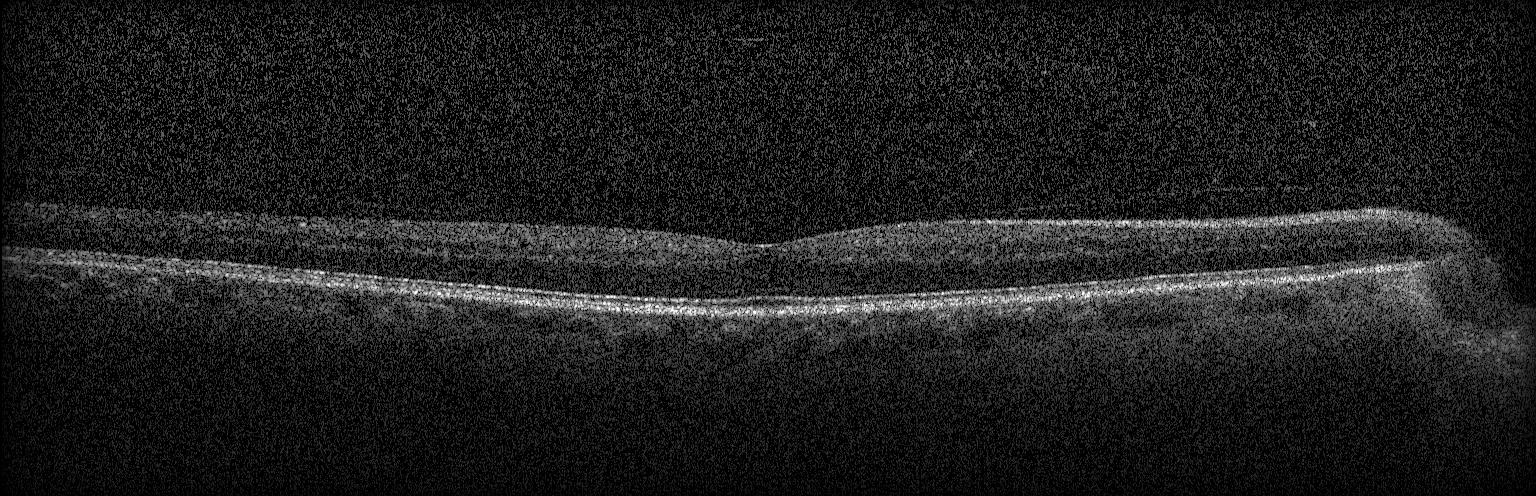
OCT B-scan · through the macula · Heidelberg Spectralis OCT system · spectral-domain OCT. Diagnosis: no evidence of choroidal neovascularization, diabetic macular edema, or drusen.